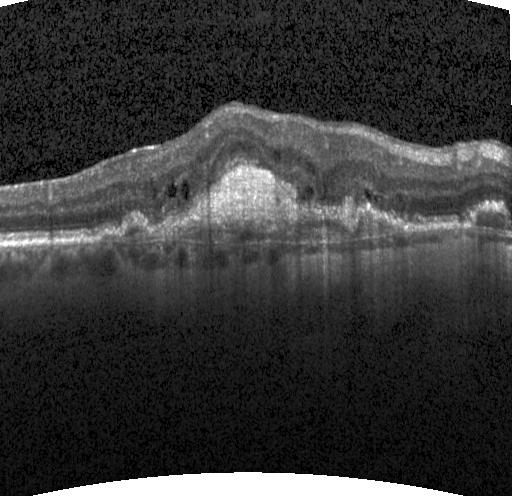

Spectral-domain OCT B-scan: choroidal neovascularization.